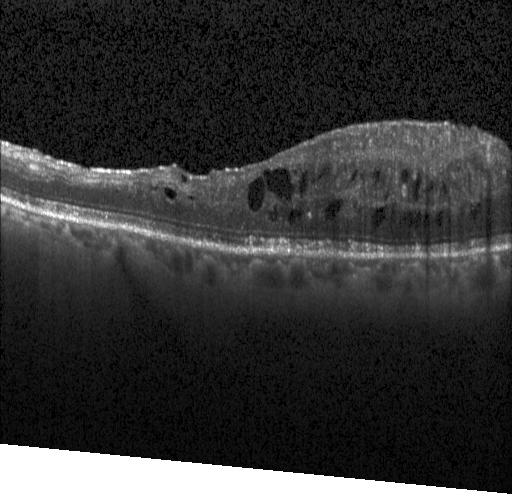 Optical coherence tomography scan · Heidelberg Spectralis · SD-OCT · horizontal scan through the fovea.
Finding: diabetic macular edema (DME).